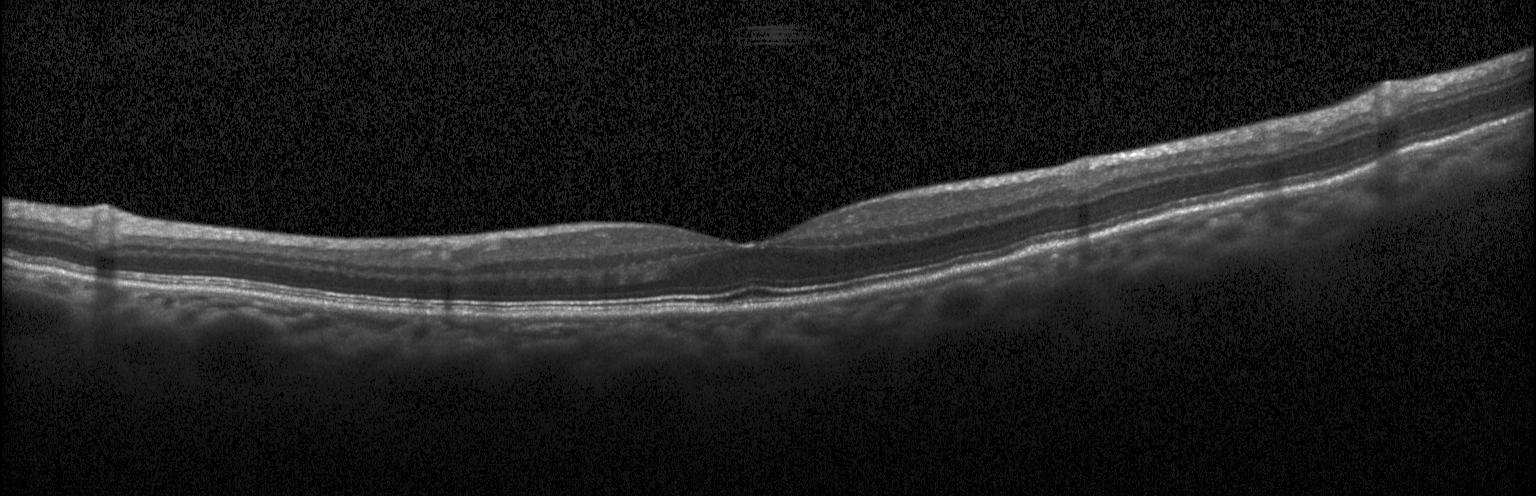
Through the macula, retinal OCT B-scan, instrument: Heidelberg Spectralis.
Impression: no CNV, DME, or drusen.